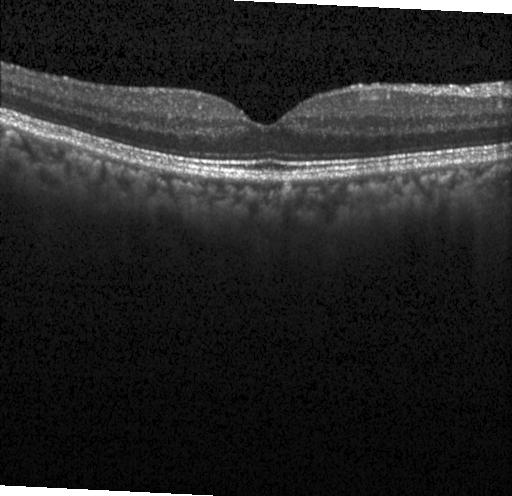
Spectral-domain OCT · Heidelberg Spectralis OCT system · optical coherence tomography scan.
Impression: no evidence of choroidal neovascularization, diabetic macular edema, or drusen.